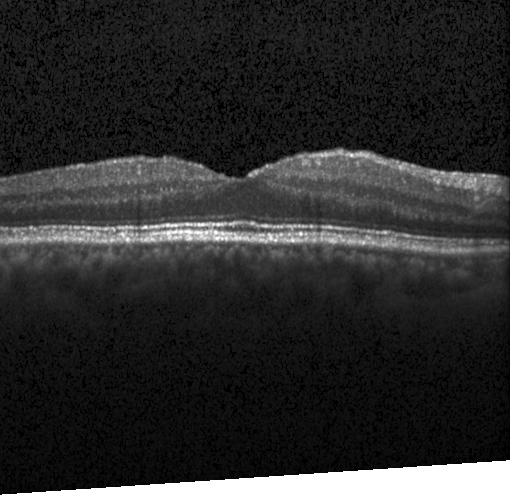

Diagnosis: no choroidal neovascularization, no diabetic macular edema, and no drusen.